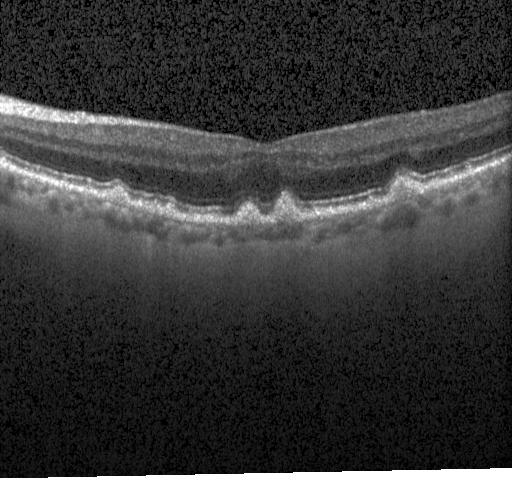 Centered on the fovea · Heidelberg Spectralis · spectral-domain optical coherence tomography · retinal OCT cross-section — The scan shows sub-RPE drusenoid deposits.